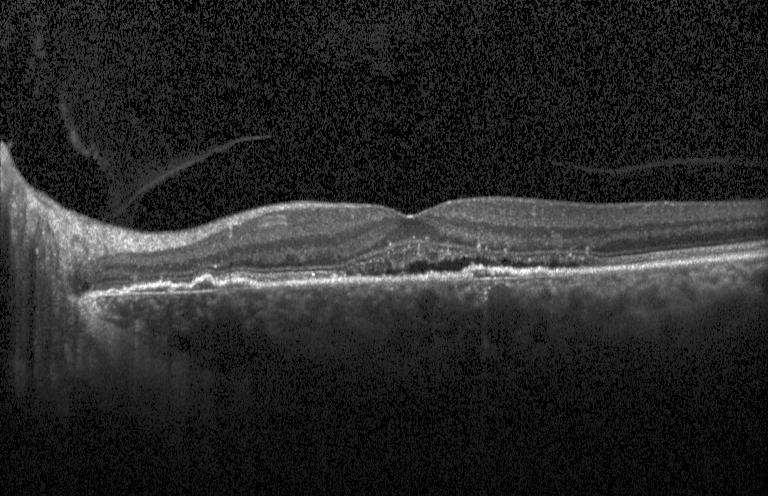 CNV.